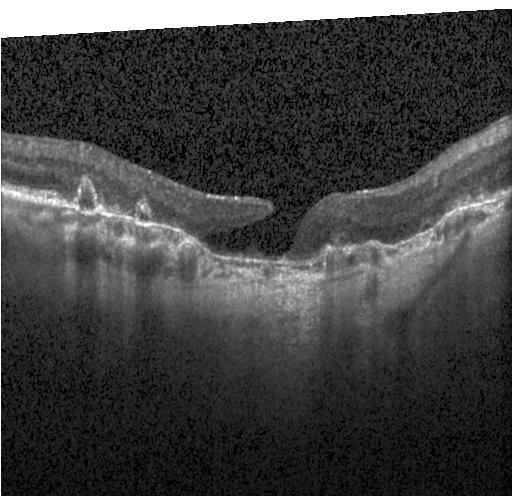 Retinal OCT B-scan. Spectral-domain optical coherence tomography. Heidelberg Spectralis OCT system. Fovea-centered. Finding: a choroidal neovascular membrane.